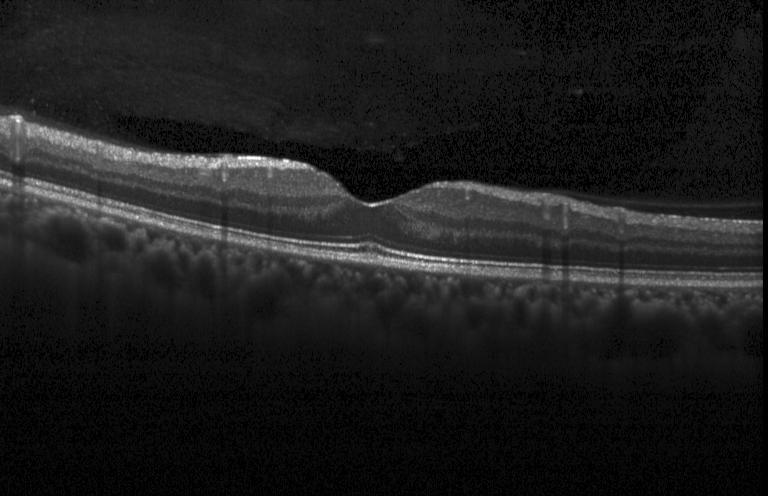
Acquired on a Heidelberg Spectralis; OCT B-scan. This B-scan demonstrates no choroidal neovascularization, diabetic macular edema, or drusen.